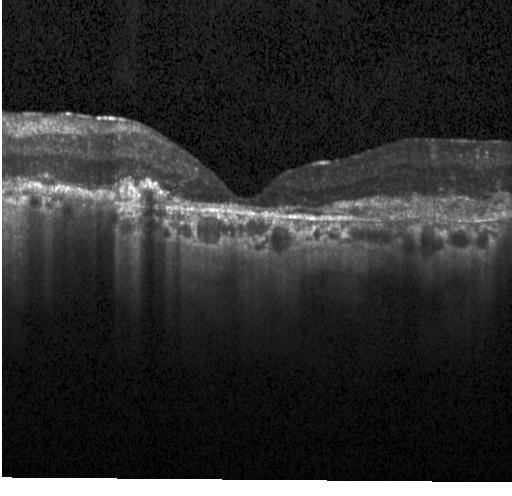 Optical coherence tomography scan
Assessment: choroidal neovascularization.